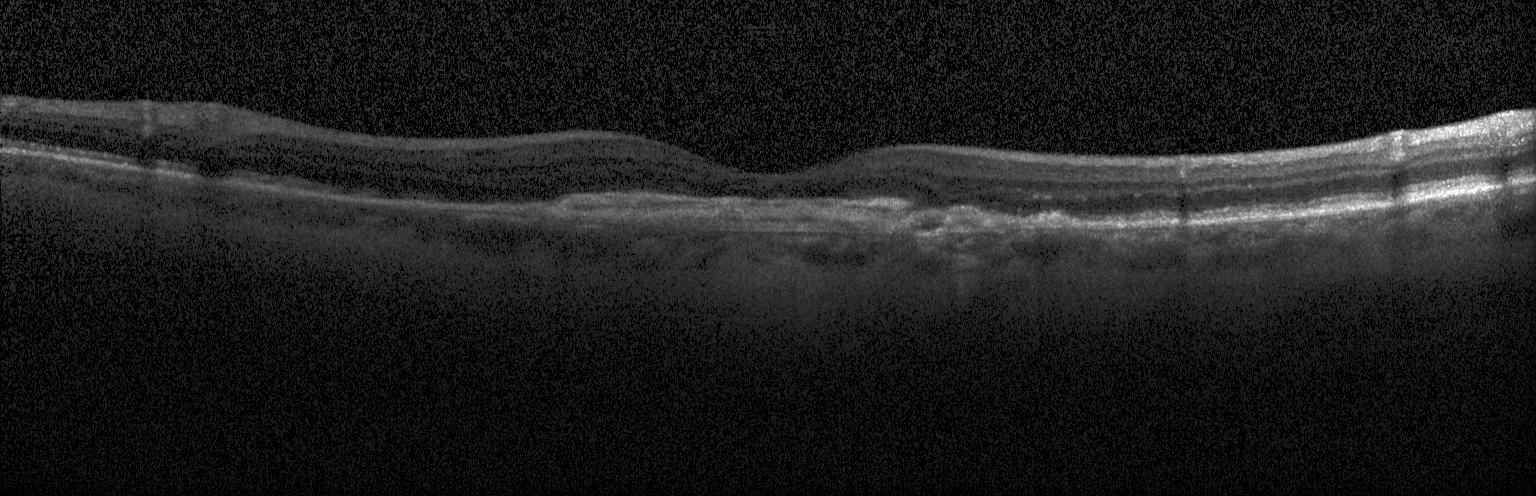
SD-OCT. Retinal OCT B-scan.
Diagnosis: choroidal neovascularization.